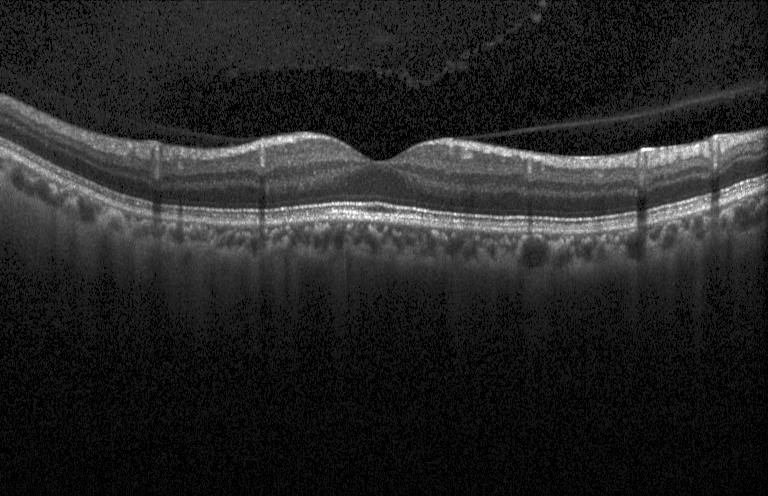 Retinal OCT cross-section
Finding: neither choroidal neovascularization, diabetic macular edema, nor drusen.